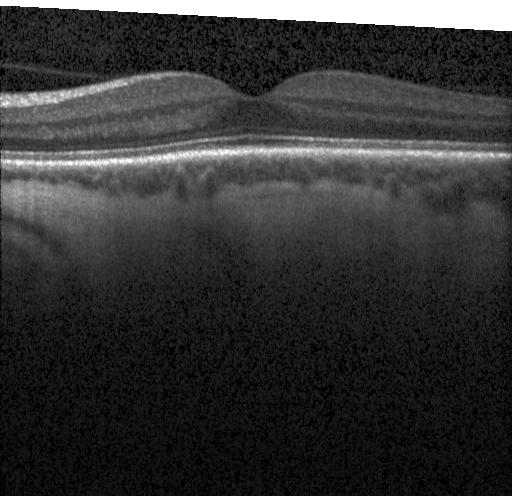
Optical coherence tomography scan, Heidelberg Spectralis, centered on the fovea. Assessment: no evidence of CNV, DME, or drusen.